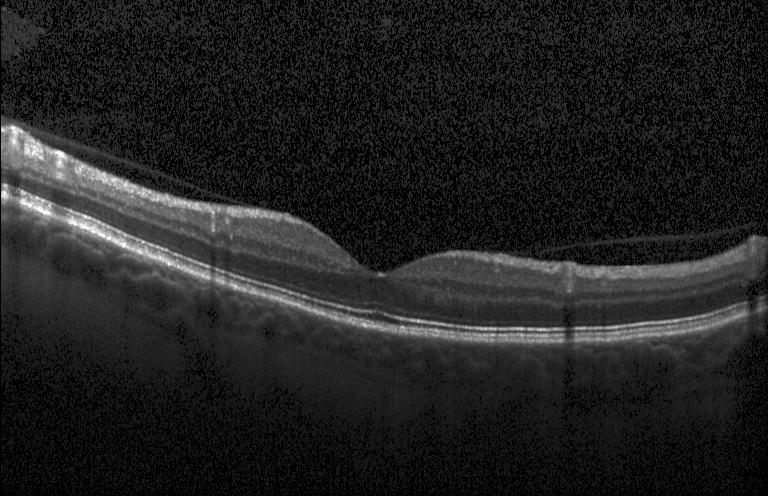

Retinal OCT cross-section — Finding: no choroidal neovascularization, diabetic macular edema, or drusen.